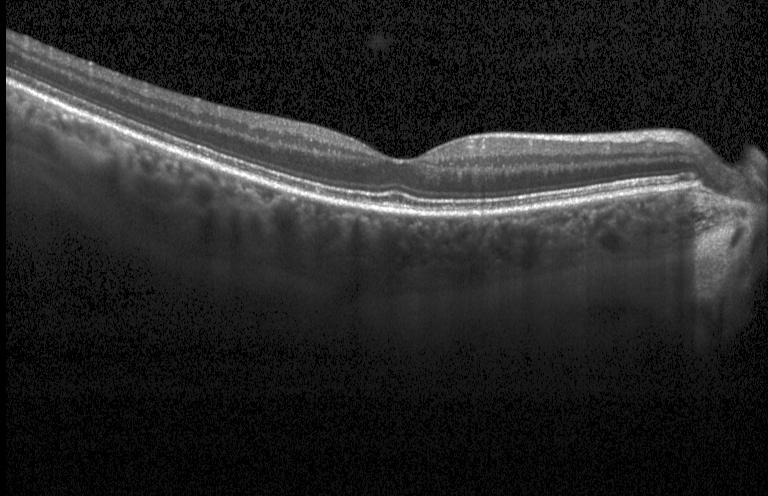

Finding: no choroidal neovascularization, diabetic macular edema, or drusen.